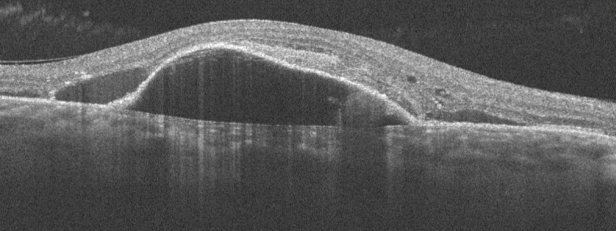
Macular scan; optical coherence tomography B-scan; instrument: Optovue Avanti RTVue XR. Impression: age-related macular degeneration (AMD).